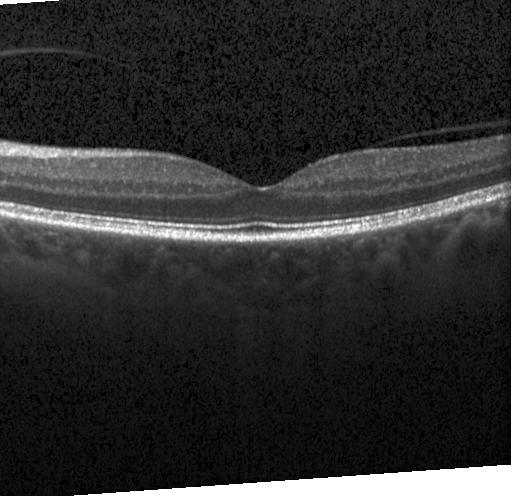

Impression: no choroidal neovascularization, diabetic macular edema, or drusen.